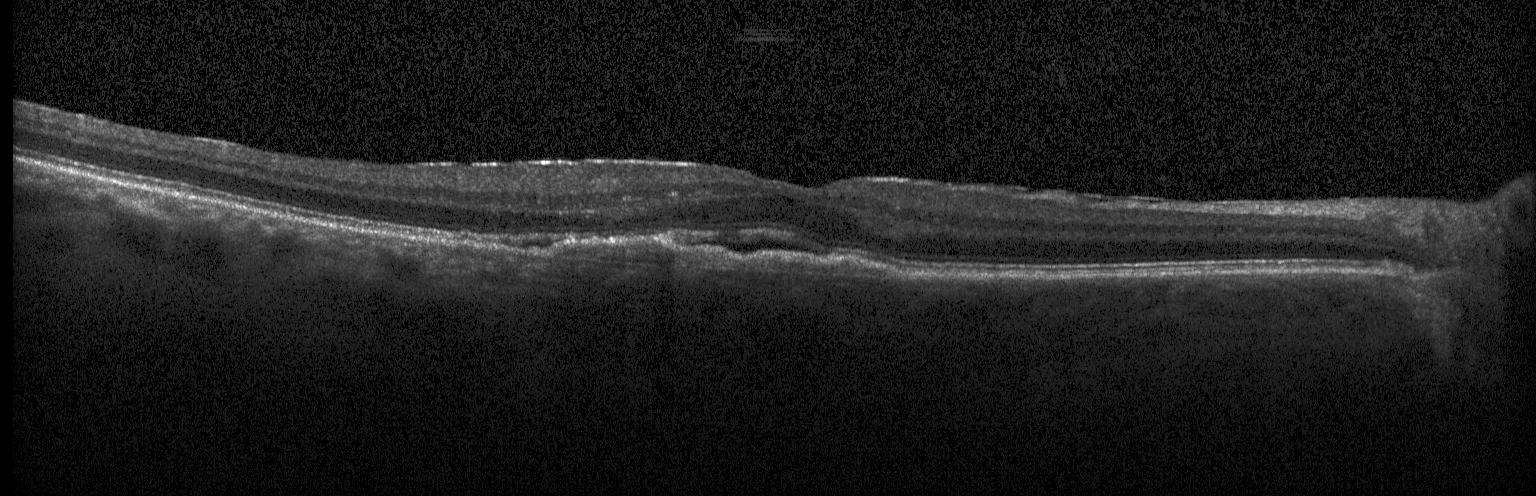

Retinal OCT B-scan — Diagnosis: a choroidal neovascular membrane.